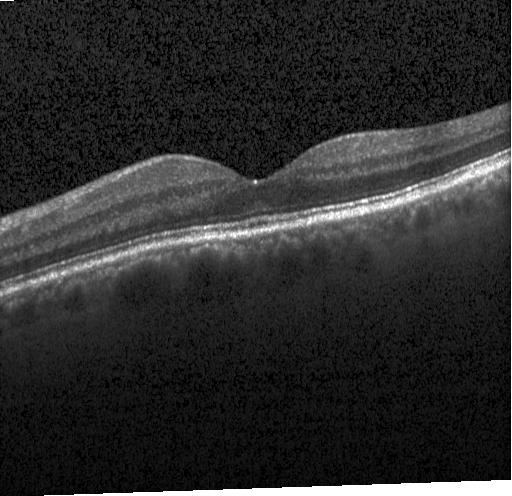 Assessment: no choroidal neovascularization, diabetic macular edema, or drusen.